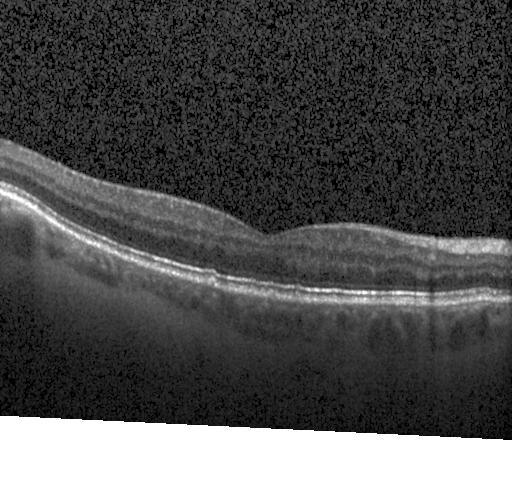
Horizontal scan through the fovea. Retinal OCT B-scan. Heidelberg Spectralis OCT system. Spectral-domain OCT
Finding: multiple drusen.